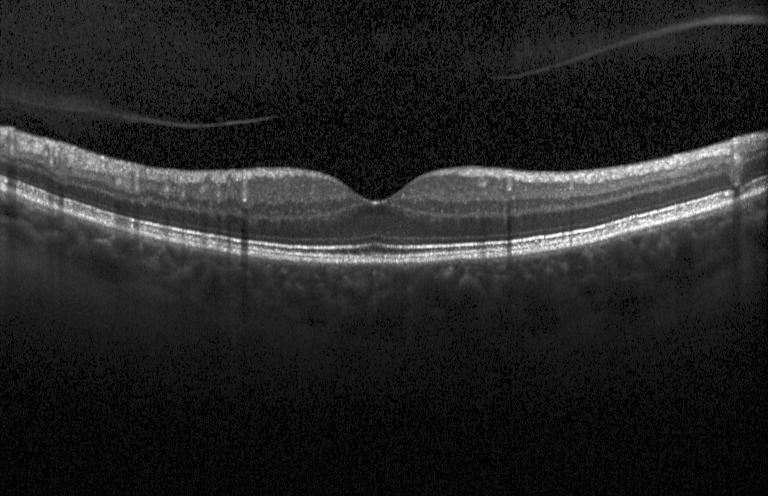

OCT scan showing no evidence of CNV, DME, or drusen.